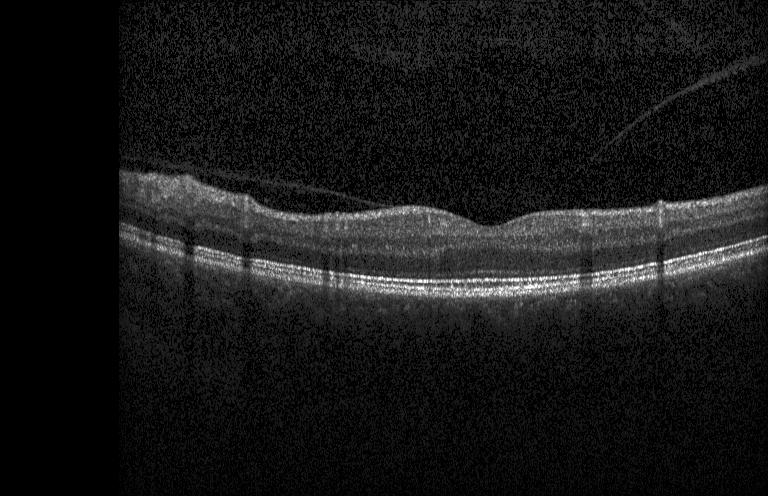

Retinal OCT cross-section showing no CNV, DME, or drusen.